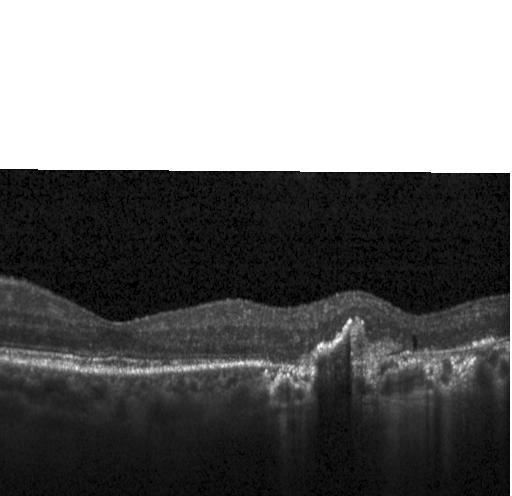 Spectral-domain OCT, through the macula, OCT line scan.
Assessment: a choroidal neovascular membrane.